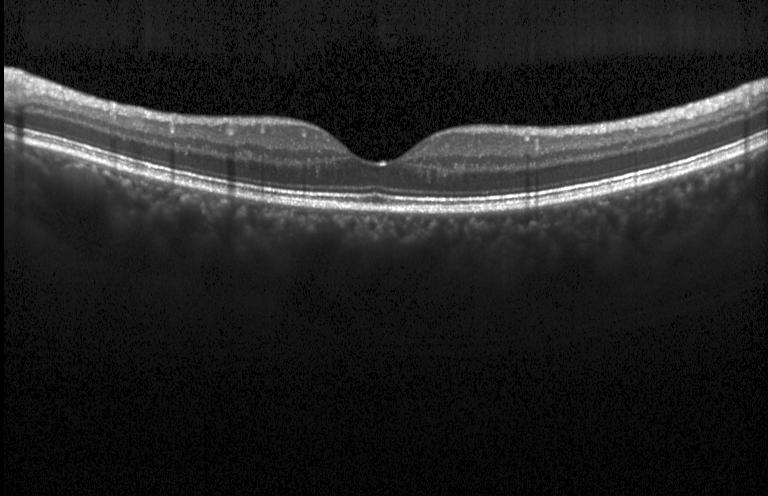
Optical coherence tomography B-scan; SD-OCT; instrument: Heidelberg Spectralis; centered on the fovea — Impression: neither choroidal neovascularization, diabetic macular edema, nor drusen.